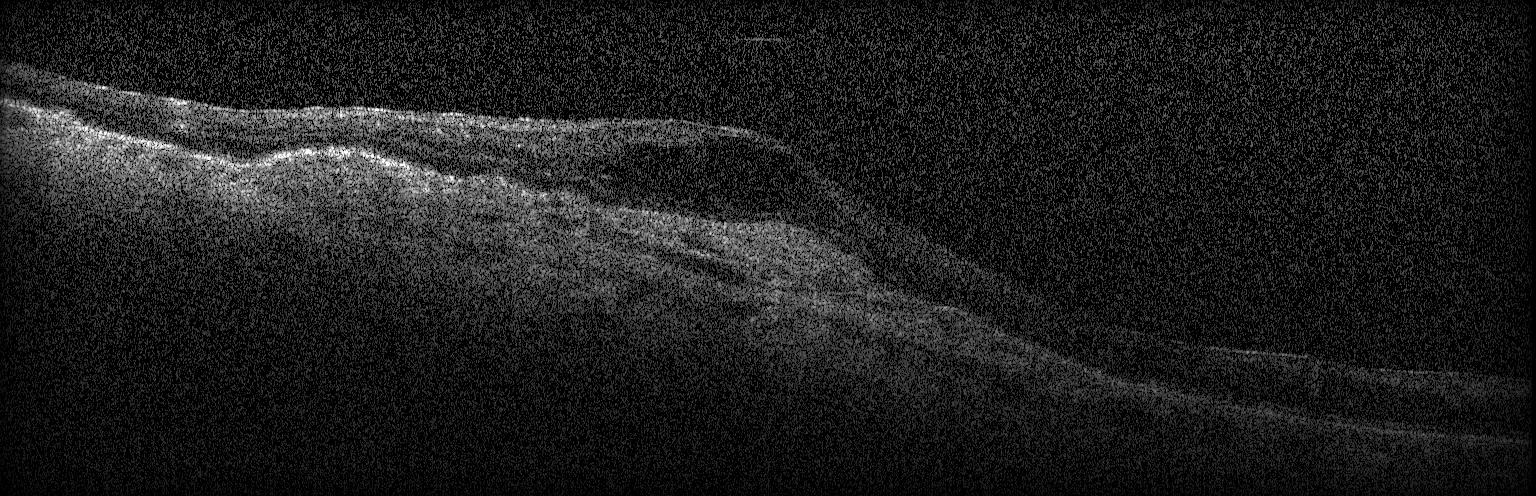

OCT B-scan, instrument: Heidelberg Spectralis. This B-scan demonstrates CNV.